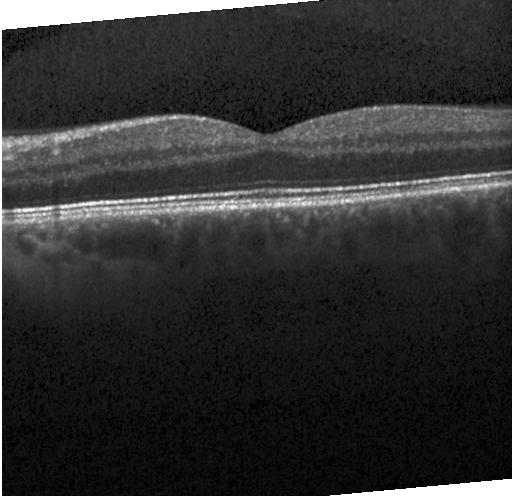 Dx: neither choroidal neovascularization, diabetic macular edema, nor drusen.